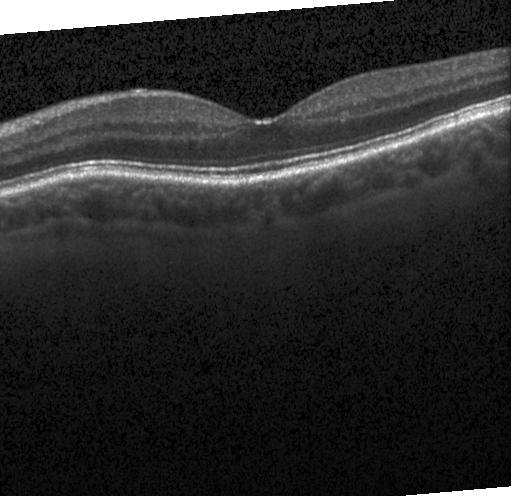

OCT B-scan showing neither CNV, DME, nor drusen.